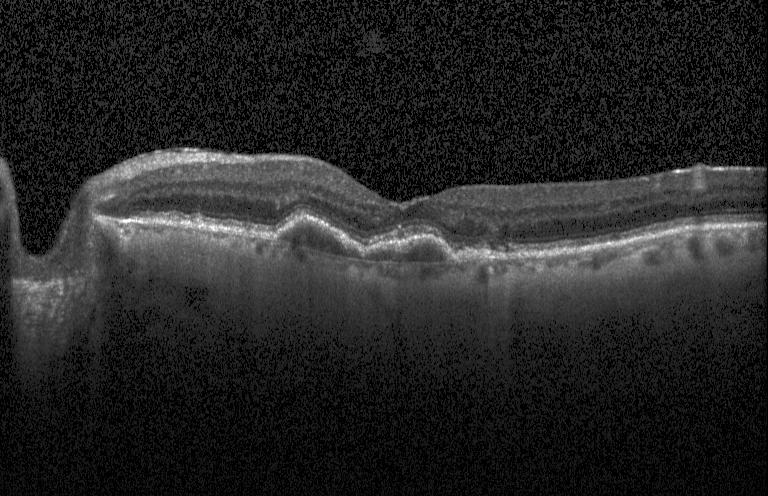

SD-OCT; through the macula; OCT line scan; acquired on a Heidelberg Spectralis.
This B-scan demonstrates choroidal neovascularization (CNV).